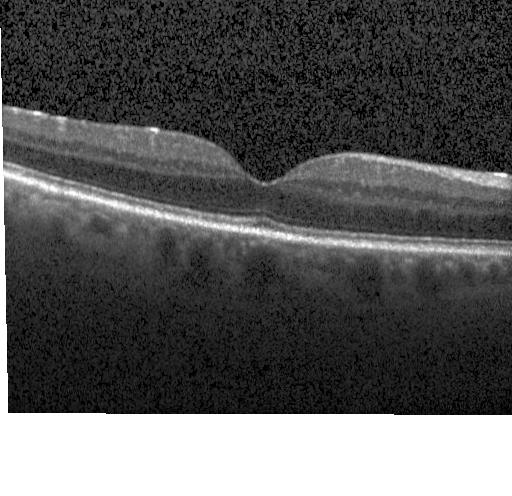

Spectral-domain optical coherence tomography · Heidelberg Spectralis OCT system · horizontal scan through the fovea · retinal OCT B-scan.
Assessment: no CNV, DME, or drusen.